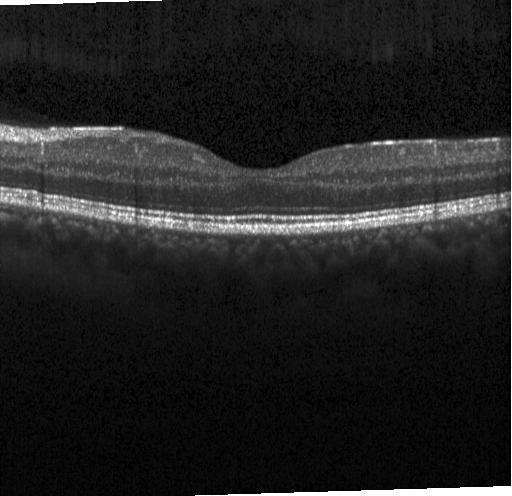

Acquired on a Heidelberg Spectralis · optical coherence tomography B-scan · centered on the fovea · SD-OCT.
Diagnosis: no evidence of choroidal neovascularization, diabetic macular edema, or drusen.